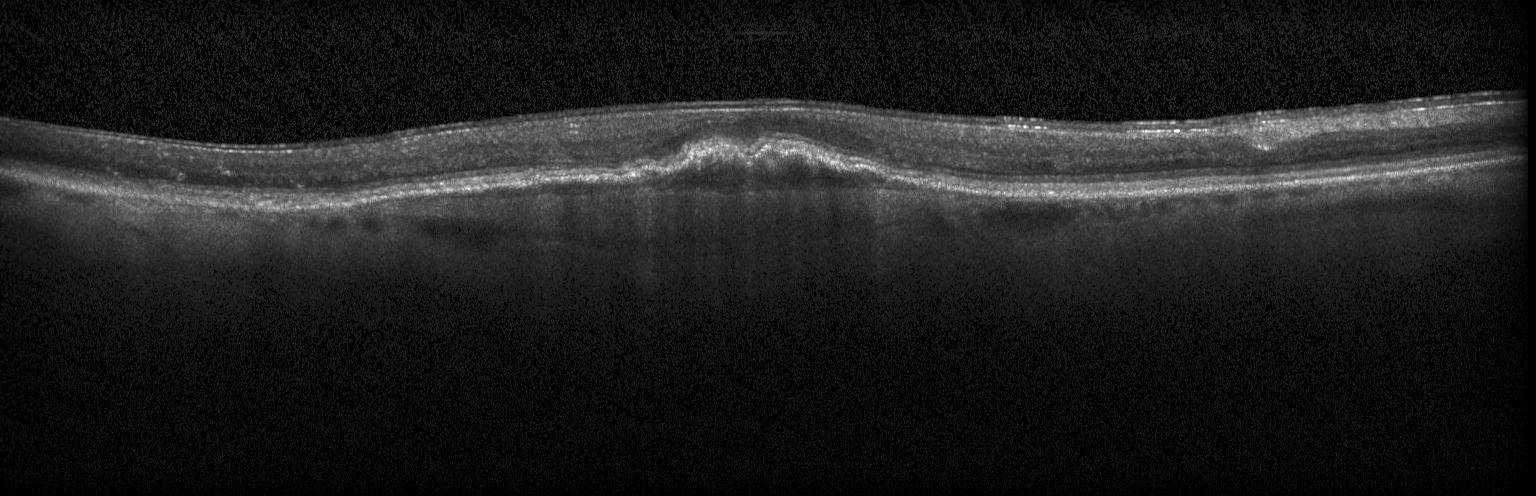
SD-OCT · Heidelberg Spectralis OCT system · optical coherence tomography B-scan. A choroidal neovascular membrane.